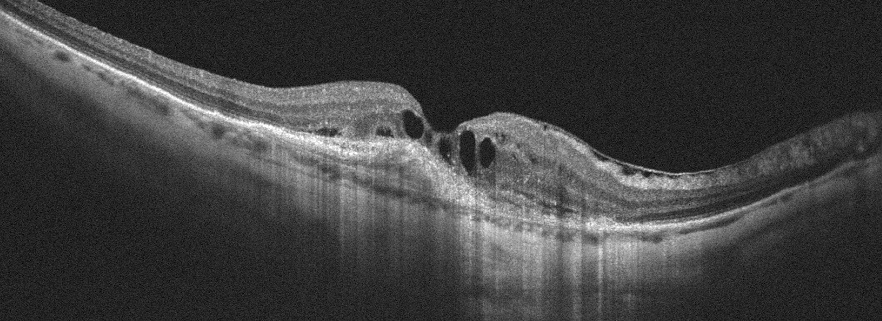

Optical coherence tomography scan. Acquired on an Optovue Avanti RTVue XR. Diagnosis: AMD.